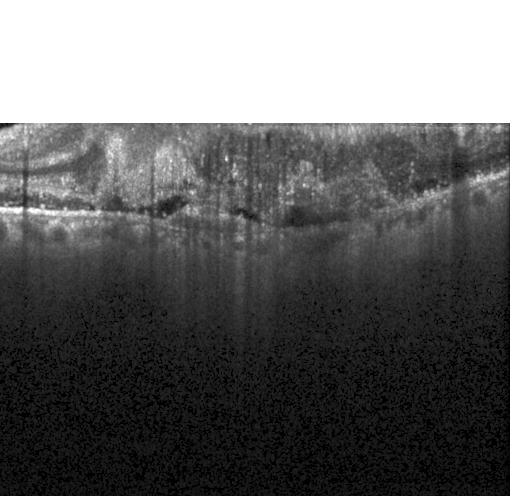 Spectral-domain OCT. OCT B-scan.
Finding: choroidal neovascularization.